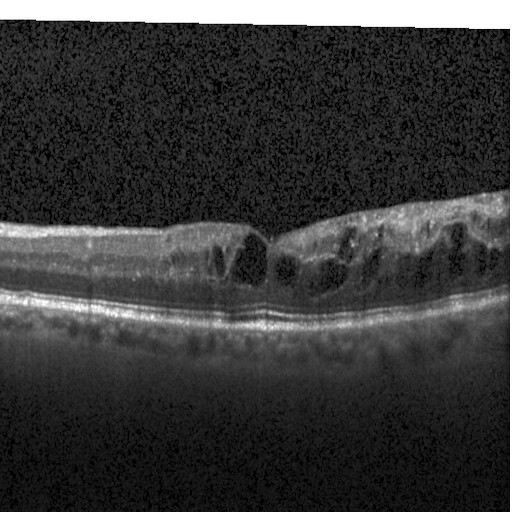 Macular OCT: diabetic macular edema.